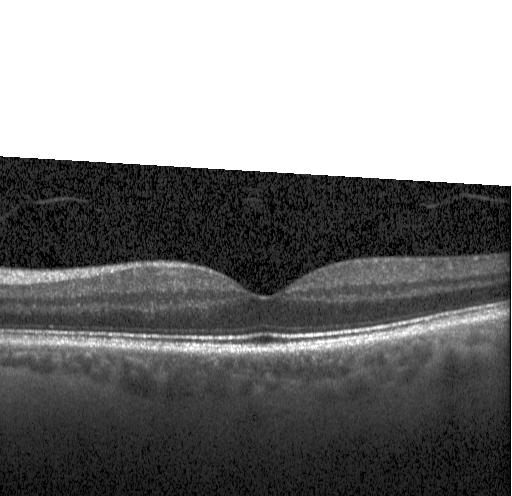 Finding: neither choroidal neovascularization, diabetic macular edema, nor drusen.